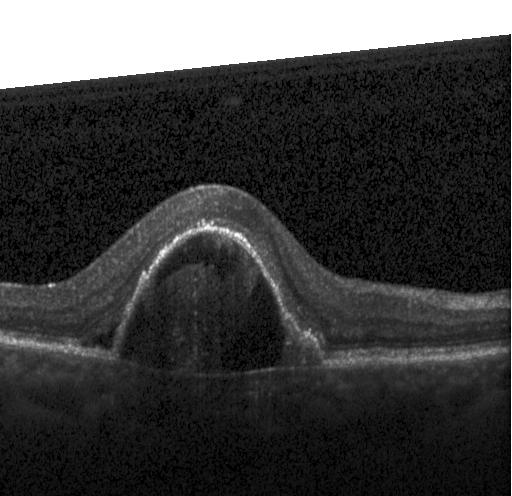
Macular OCT: choroidal neovascularization (CNV).